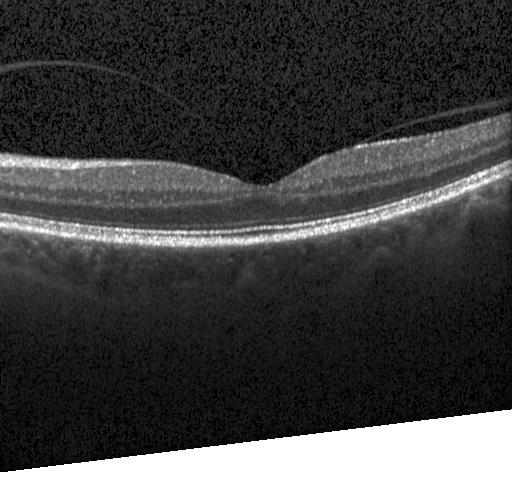
SD-OCT. OCT B-scan.
Neither CNV, DME, nor drusen.